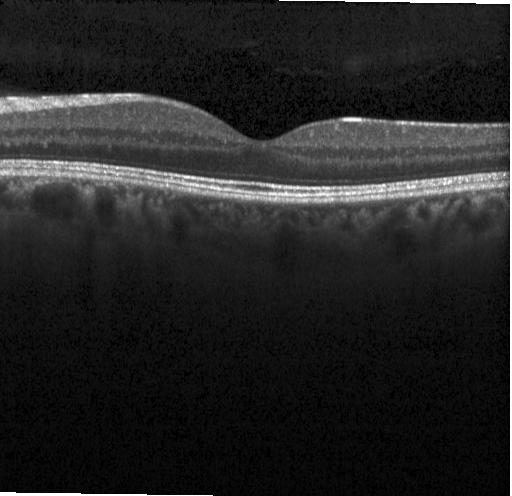
Optical coherence tomography scan.
Impression: no choroidal neovascularization, no diabetic macular edema, and no drusen.